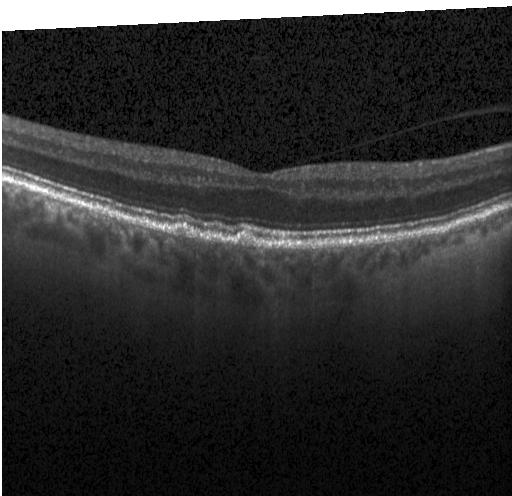

Through the macula · spectral-domain OCT · optical coherence tomography scan · instrument: Heidelberg Spectralis
Impression: multiple drusen.